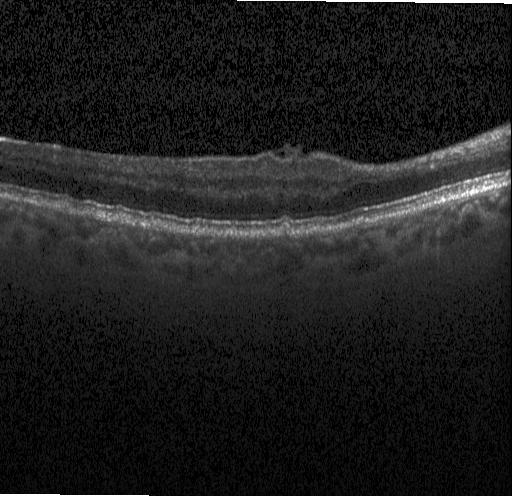
Spectral-domain optical coherence tomography, optical coherence tomography scan — Impression: drusen.